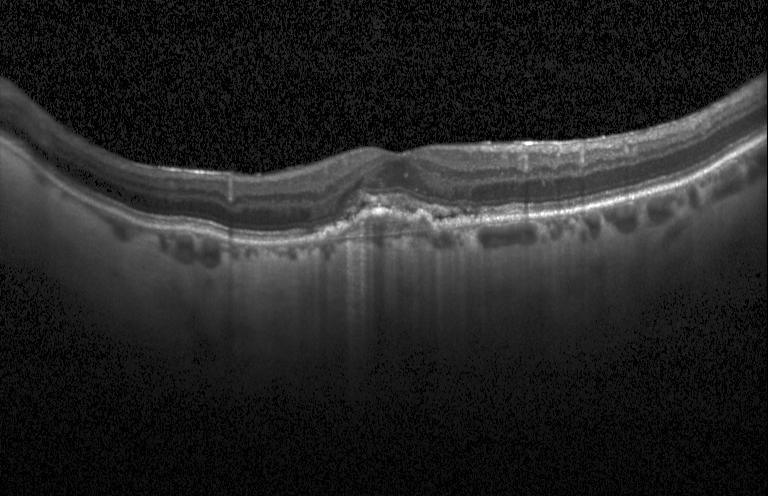
Retinal OCT cross-section — This B-scan demonstrates a choroidal neovascular membrane.